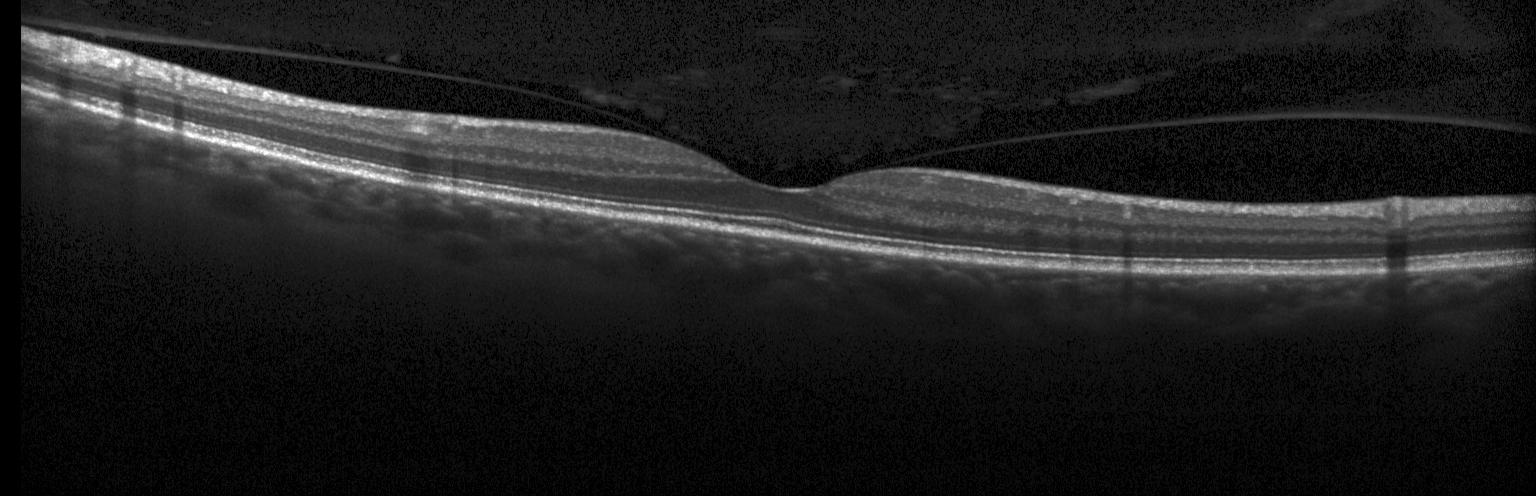 OCT B-scan · spectral-domain OCT — OCT finding: neither choroidal neovascularization, diabetic macular edema, nor drusen.